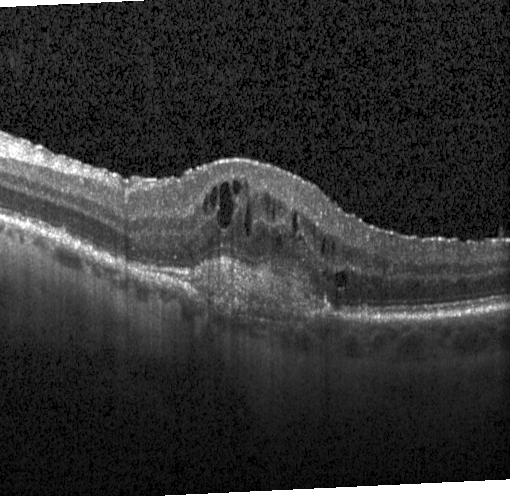

OCT line scan — Assessment: a choroidal neovascular membrane.